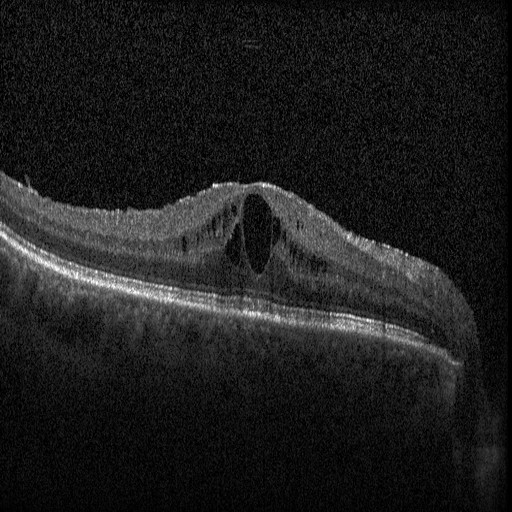 Optical coherence tomography B-scan.
Diagnosis: diabetic macular edema (DME).